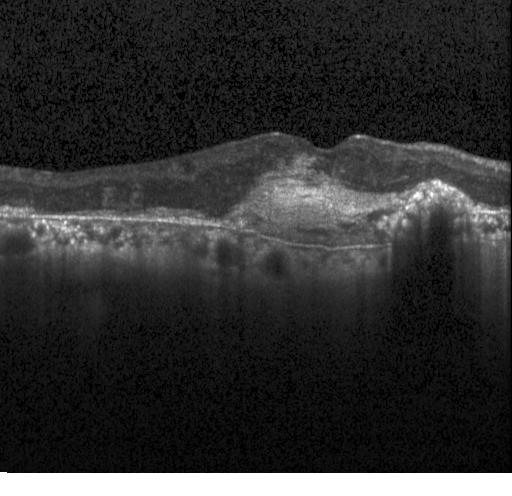 Retinal OCT cross-section. Heidelberg Spectralis. Spectral-domain OCT
Assessment: a choroidal neovascular membrane.